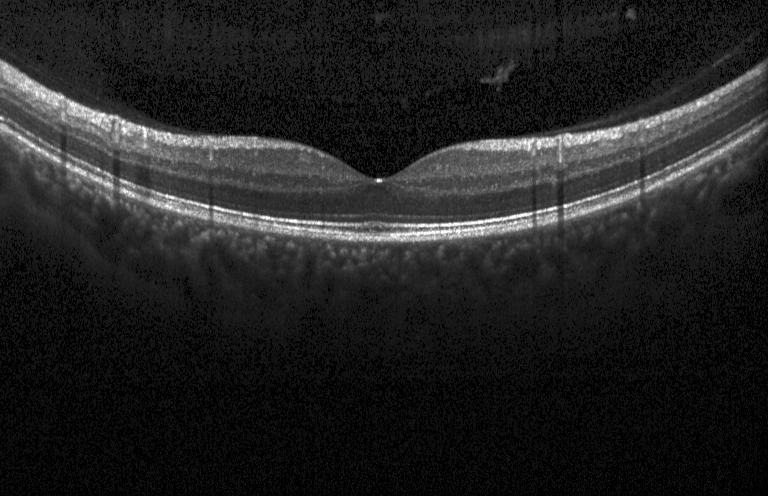 Heidelberg Spectralis. Spectral-domain optical coherence tomography. Optical coherence tomography B-scan — Impression: no choroidal neovascularization, no diabetic macular edema, and no drusen.